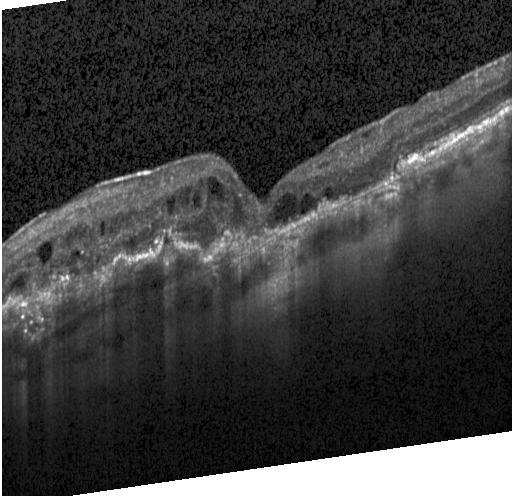

Fovea-centered; acquired on a Heidelberg Spectralis; spectral-domain optical coherence tomography; retinal OCT cross-section
Finding: choroidal neovascularization (CNV).